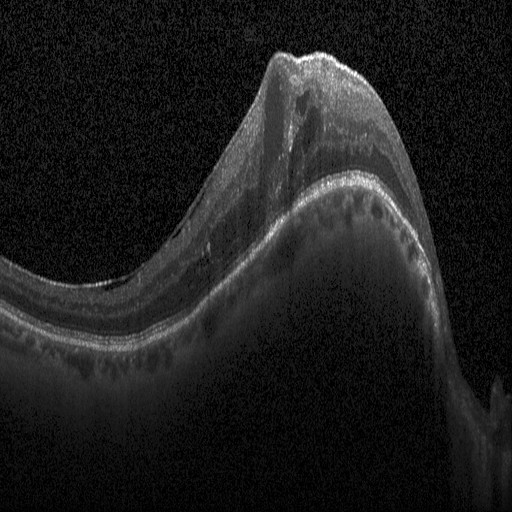

OCT line scan, Heidelberg Spectralis
Diagnosis: DME.